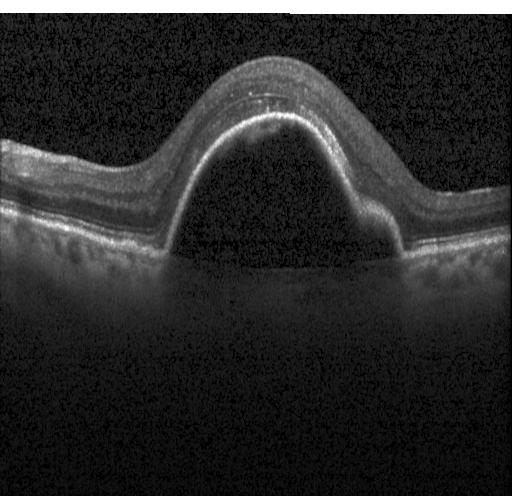
Macular OCT: choroidal neovascularization.